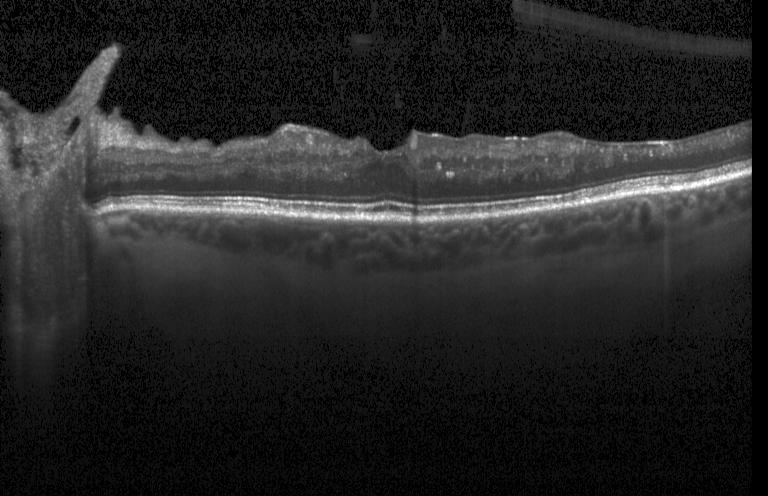 Diabetic macular edema.